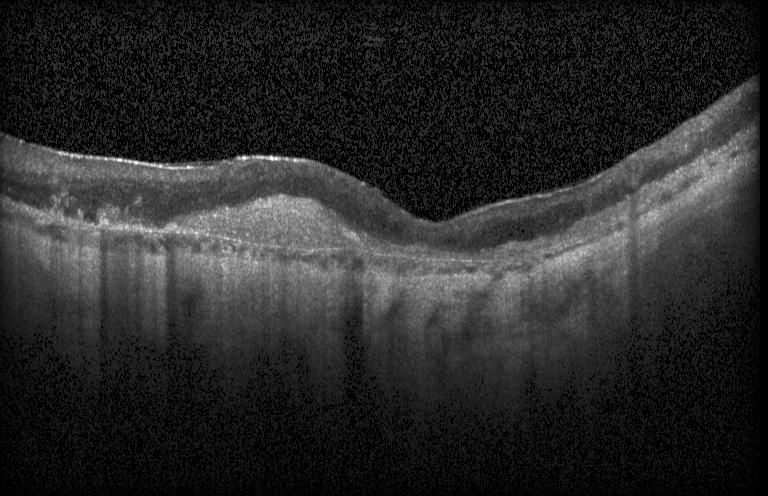
Heidelberg Spectralis OCT system, OCT line scan, through the macula. The scan shows CNV.